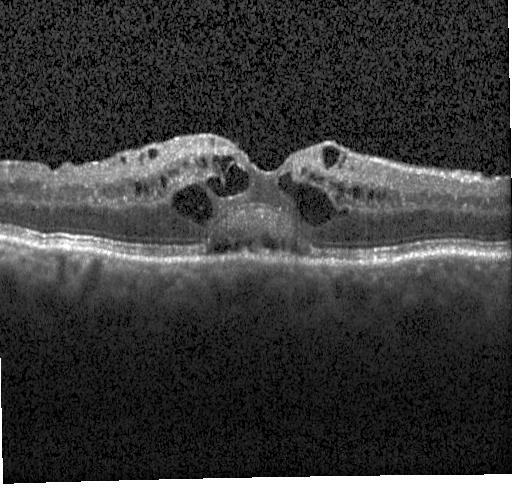
Retinal OCT B-scan, spectral-domain optical coherence tomography, macular scan, instrument: Heidelberg Spectralis.
Macular OCT: diabetic macular edema.